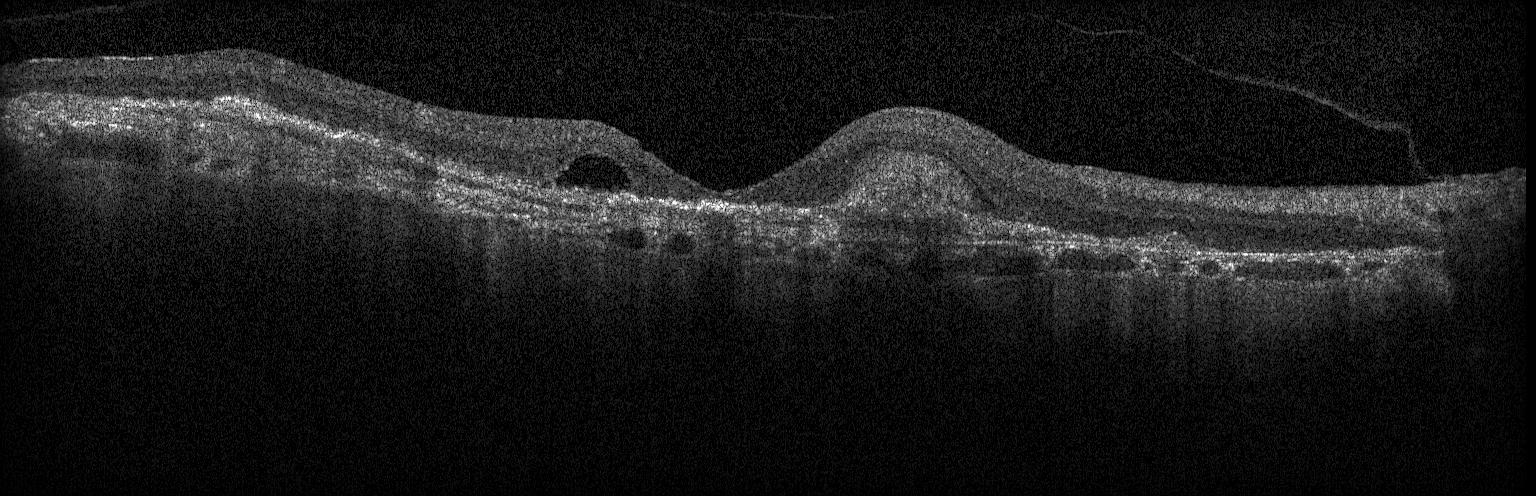
Impression: a choroidal neovascular membrane.